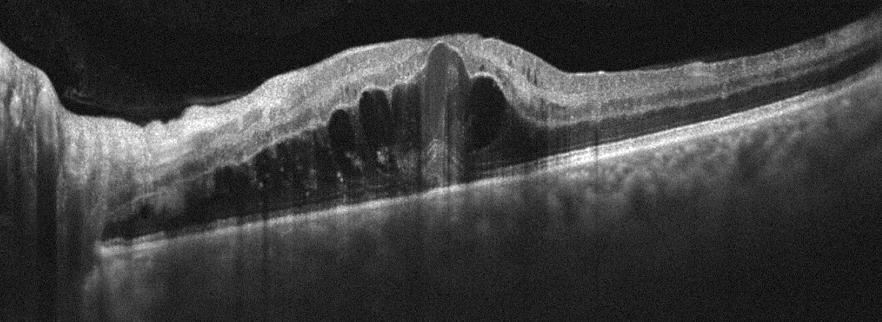

Optical coherence tomography scan. This B-scan demonstrates retinal vein occlusion (RVO).